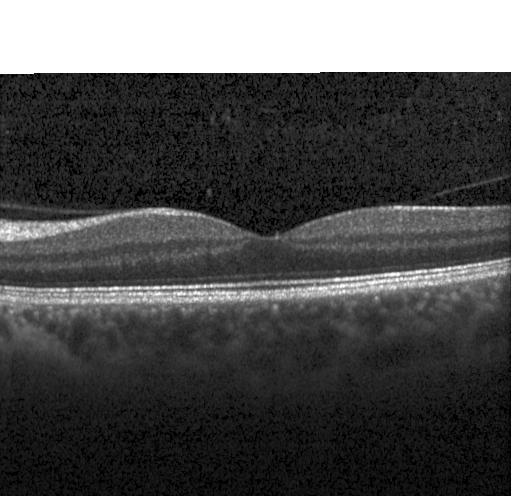
OCT B-scan; spectral-domain optical coherence tomography — This B-scan demonstrates no choroidal neovascularization, no diabetic macular edema, and no drusen.